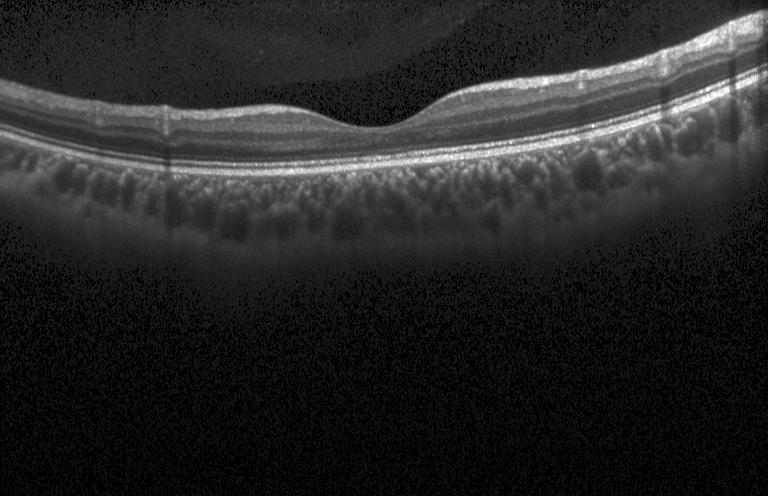
OCT scan showing neither choroidal neovascularization, diabetic macular edema, nor drusen.